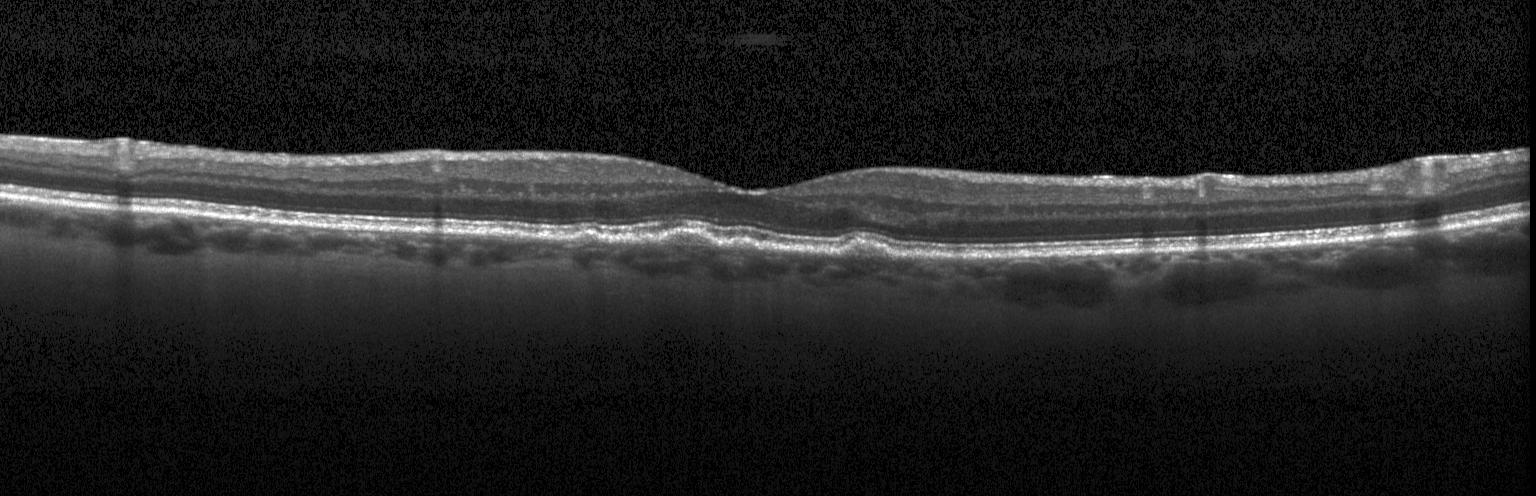

Impression: sub-RPE drusenoid deposits.